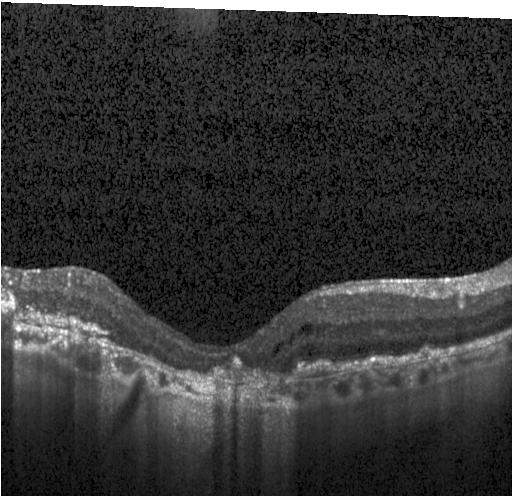
Spectral-domain OCT; retinal OCT B-scan.
Dx: choroidal neovascularization.